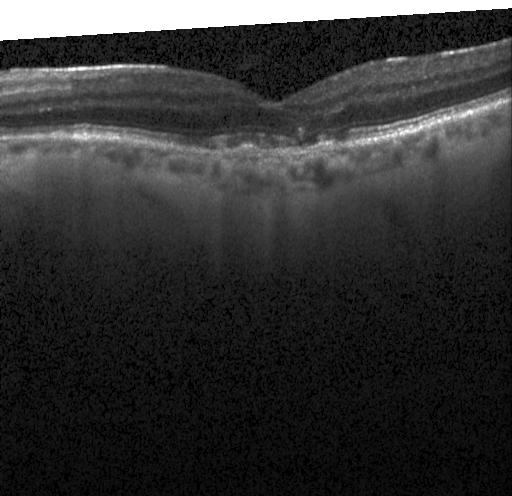 Instrument: Heidelberg Spectralis. Spectral-domain optical coherence tomography. Retinal OCT B-scan. Horizontal scan through the fovea. Impression: choroidal neovascularization.